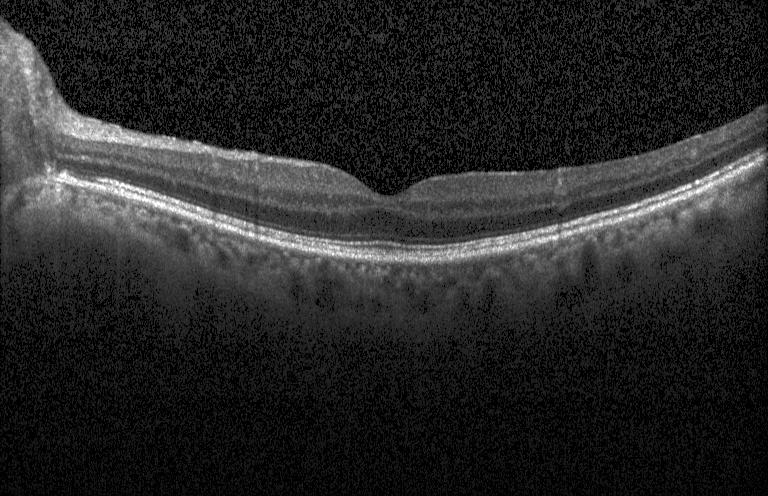 SD-OCT. OCT B-scan. Instrument: Heidelberg Spectralis. Fovea-centered
This B-scan demonstrates no CNV, DME, or drusen.